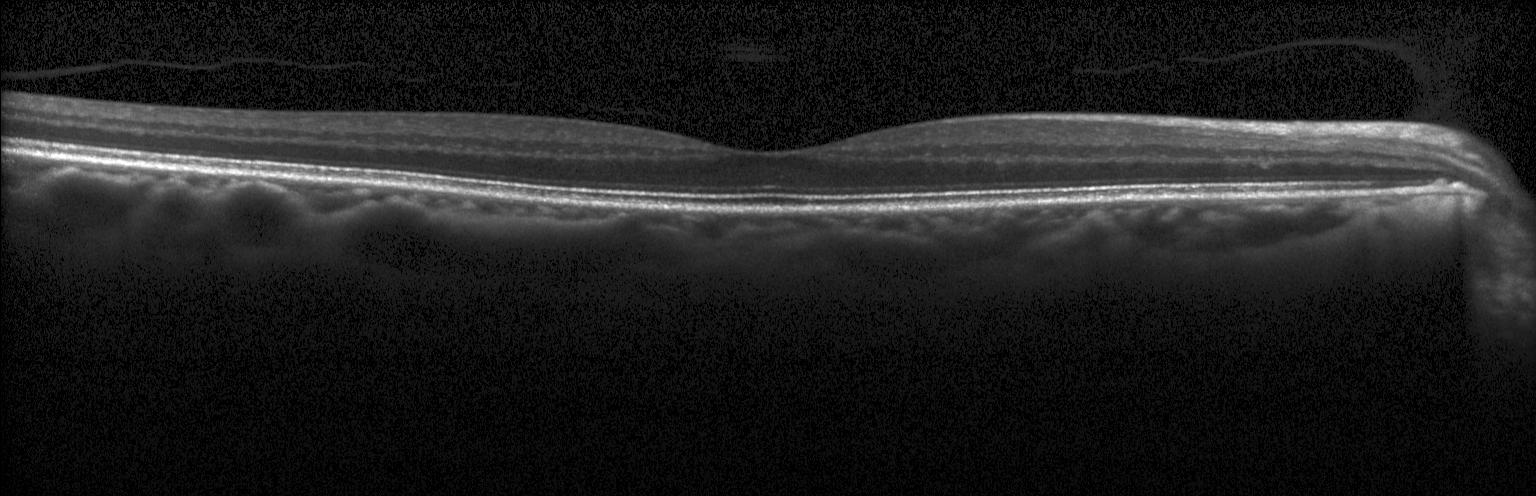

Spectral-domain OCT B-scan: no evidence of choroidal neovascularization, diabetic macular edema, or drusen.